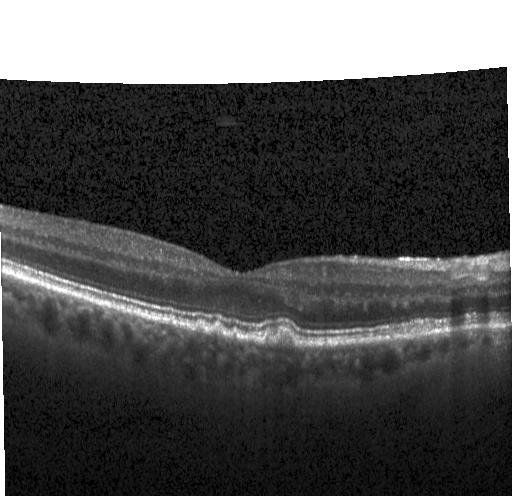

Optical coherence tomography B-scan — This B-scan demonstrates sub-RPE drusenoid deposits.